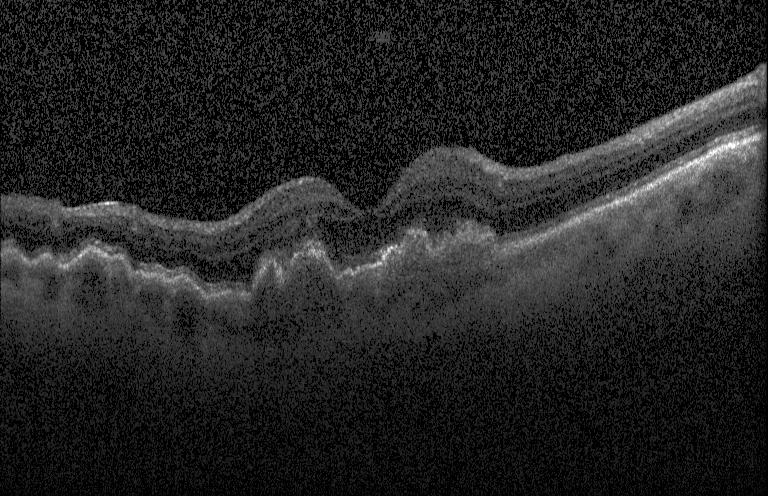
Instrument: Heidelberg Spectralis, macular scan, retinal OCT B-scan.
Diagnosis: a choroidal neovascular membrane.